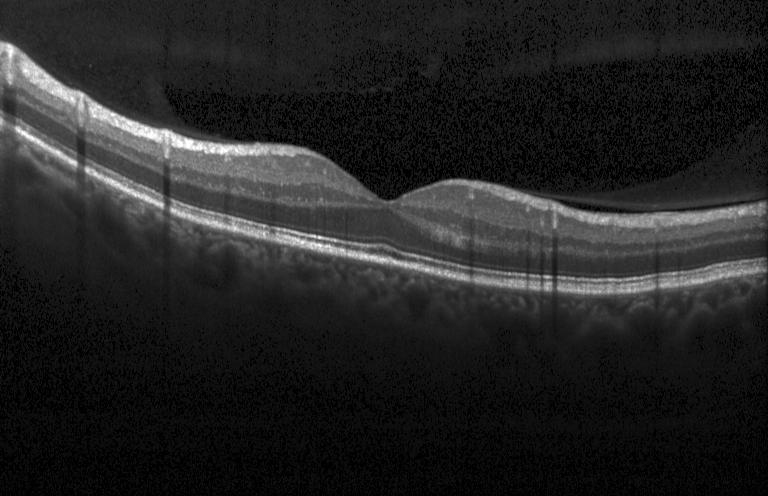 This B-scan demonstrates neither choroidal neovascularization, diabetic macular edema, nor drusen.